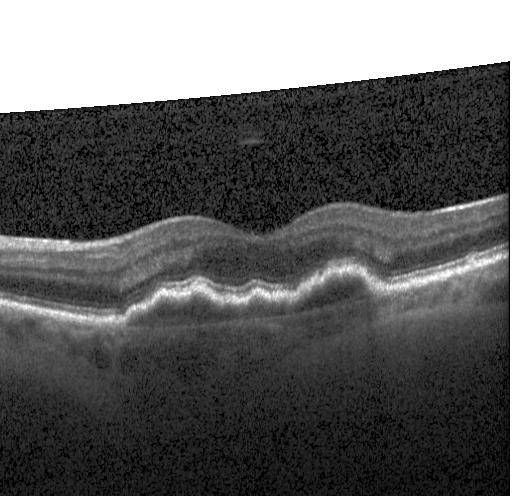

Spectral-domain OCT B-scan: choroidal neovascularization.